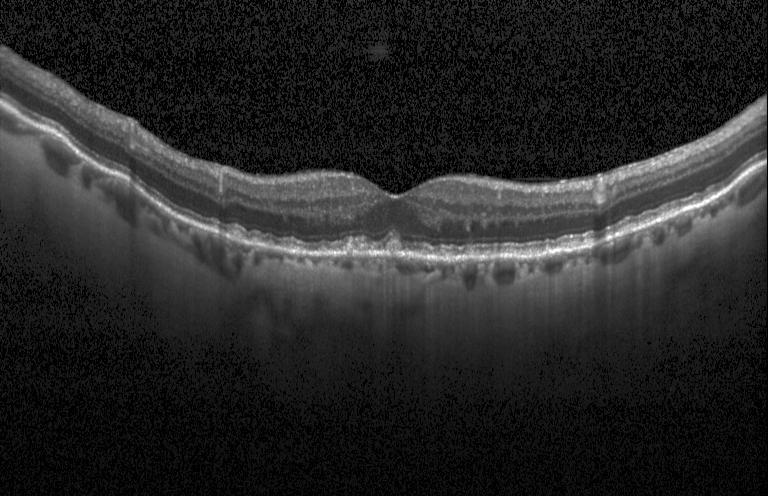 Centered on the fovea · acquired on a Heidelberg Spectralis · optical coherence tomography scan.
Macular OCT: sub-RPE drusenoid deposits.